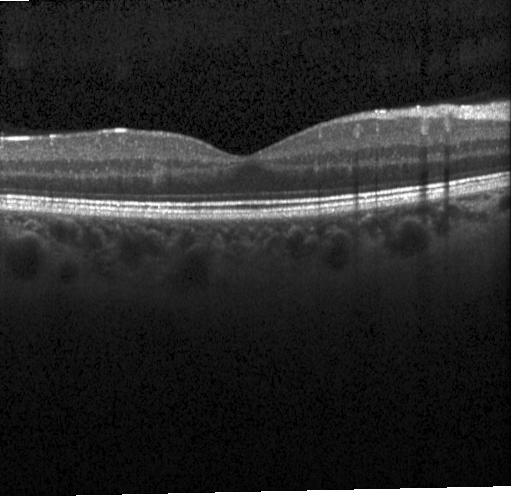
Spectral-domain OCT, instrument: Heidelberg Spectralis, OCT line scan — Diagnosis: no CNV, no DME, and no drusen.